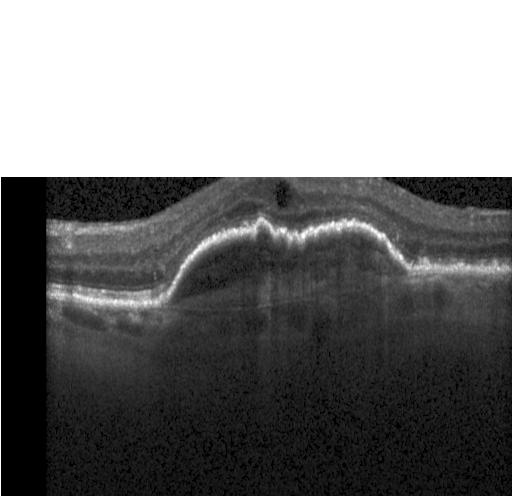
Optical coherence tomography scan · through the macula · Heidelberg Spectralis OCT system · spectral-domain optical coherence tomography. OCT finding: a choroidal neovascular membrane.